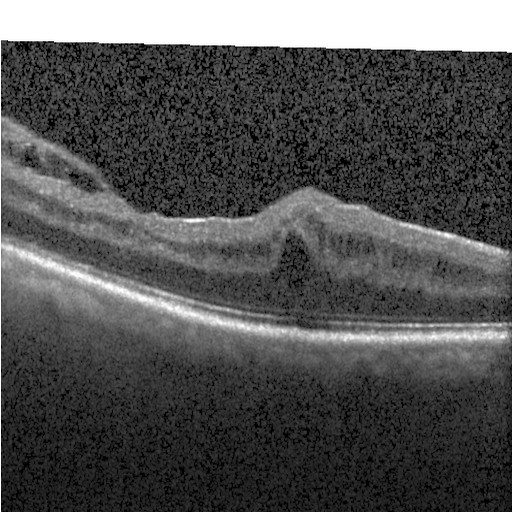 SD-OCT; fovea-centered; optical coherence tomography scan; Heidelberg Spectralis OCT system
Dx: diabetic macular edema (DME).